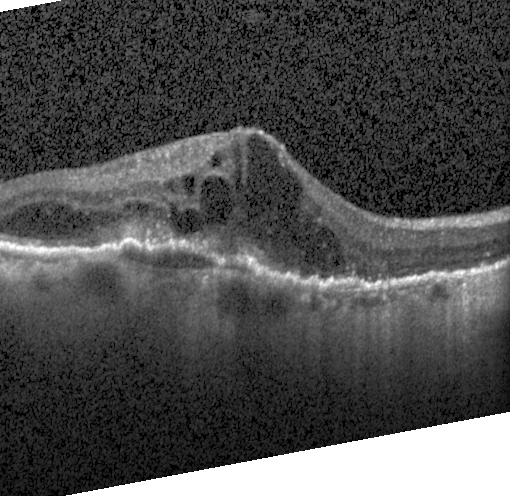
Optical coherence tomography scan. Finding: a choroidal neovascular membrane.